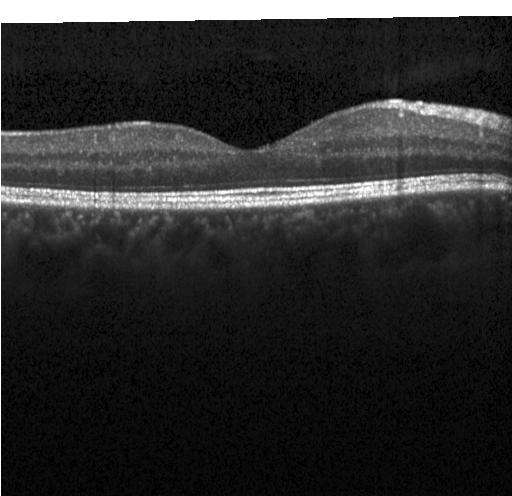

Macular OCT demonstrating no evidence of choroidal neovascularization, diabetic macular edema, or drusen.